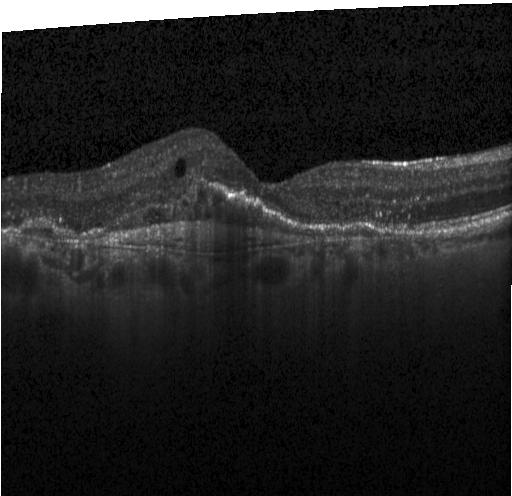 Retinal OCT cross-section showing a choroidal neovascular membrane.